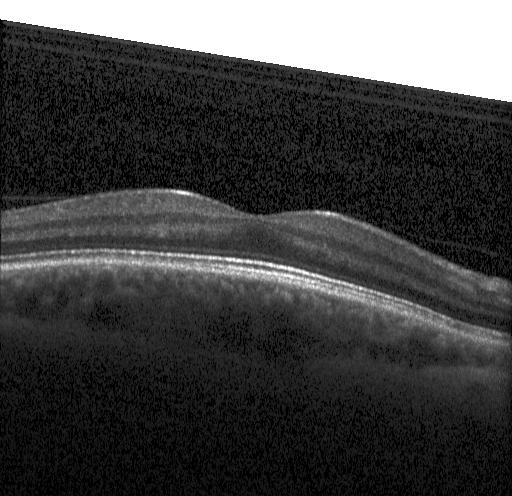

SD-OCT, retinal OCT B-scan, Heidelberg Spectralis. Neither choroidal neovascularization, diabetic macular edema, nor drusen.